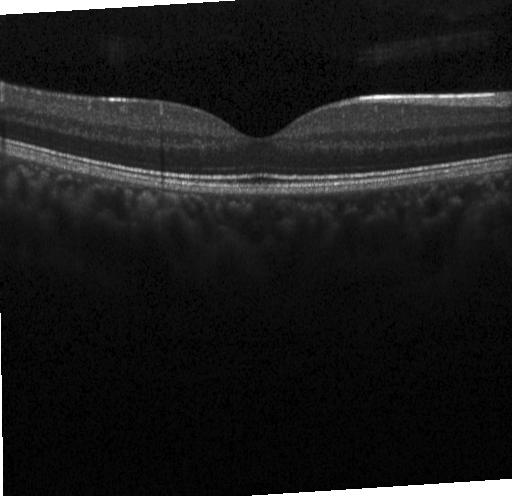 OCT line scan · Heidelberg Spectralis OCT system — Assessment: no CNV, no DME, and no drusen.